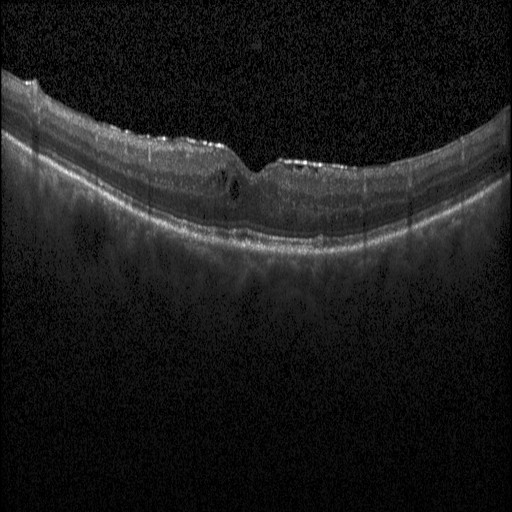 Retinal OCT cross-section
Finding: DME.